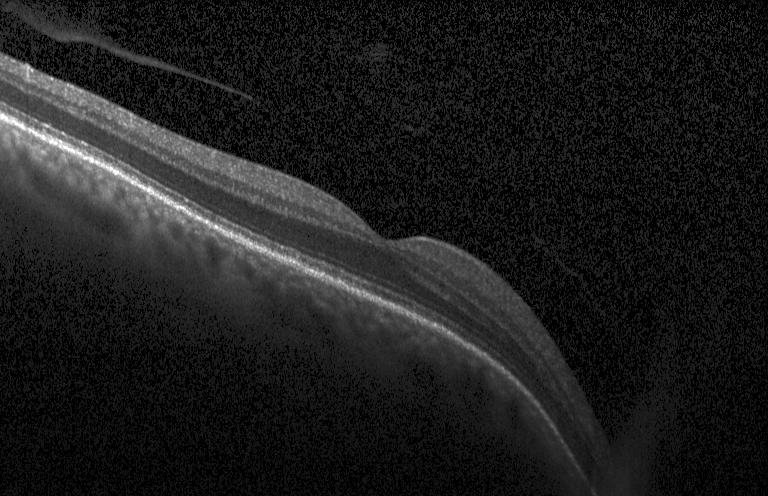 Finding: no evidence of choroidal neovascularization, diabetic macular edema, or drusen.